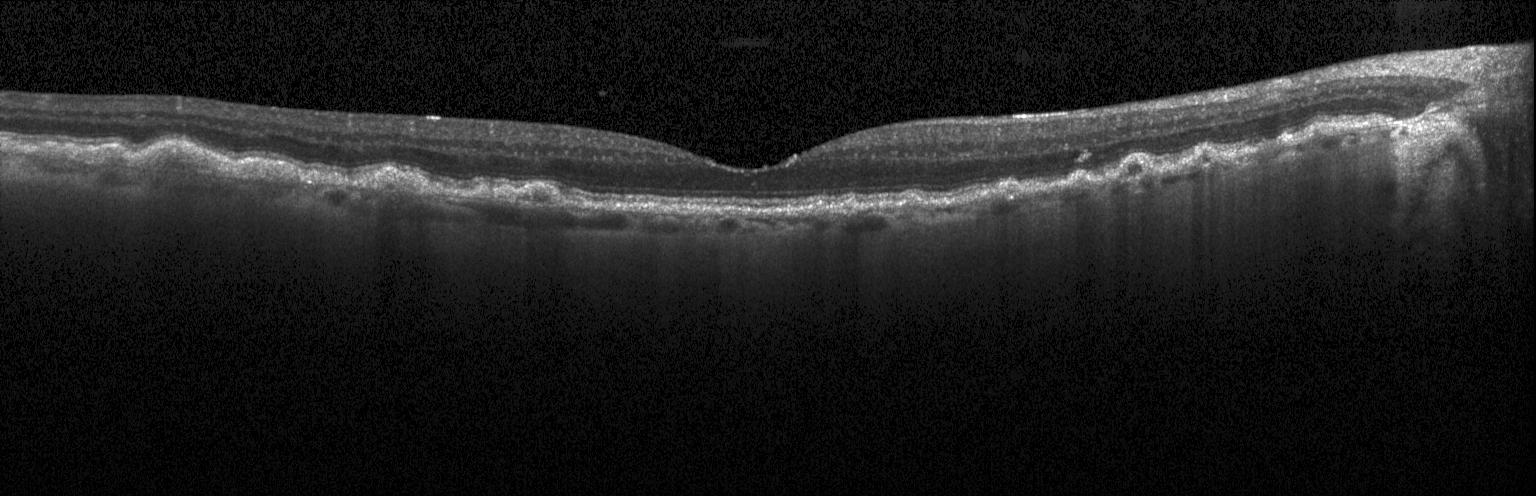 OCT B-scan. Finding: drusen.